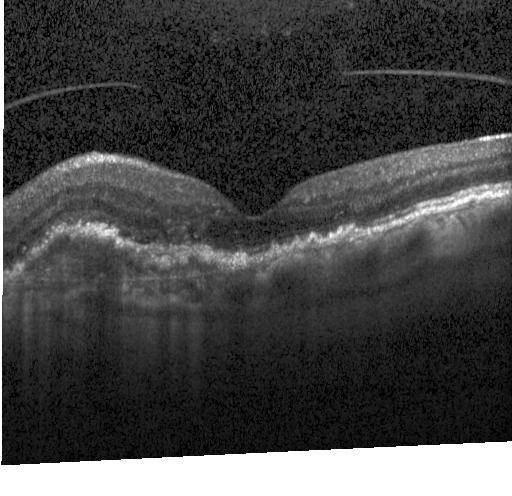

Spectral-domain optical coherence tomography, fovea-centered, OCT line scan, Heidelberg Spectralis OCT system
Diagnosis: a choroidal neovascular membrane.